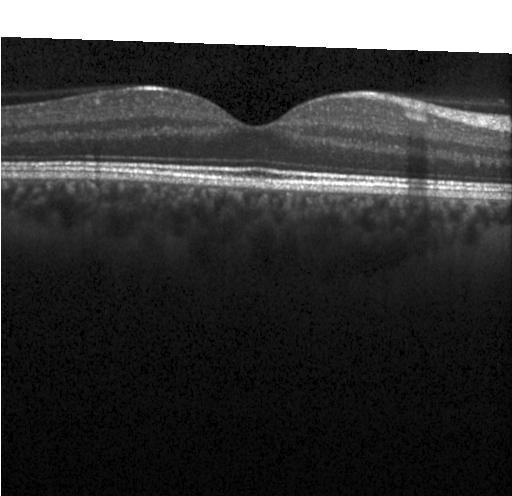
The scan shows no evidence of choroidal neovascularization, diabetic macular edema, or drusen.